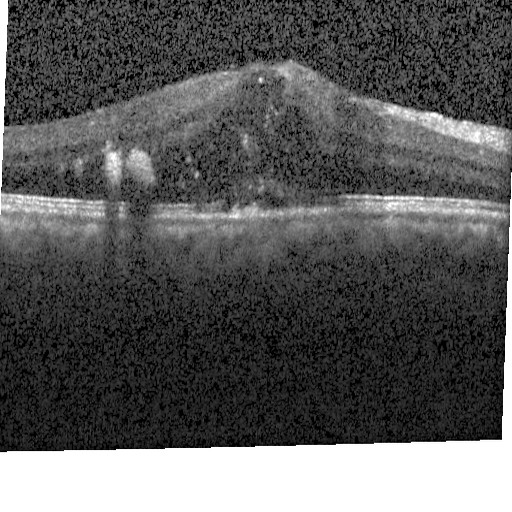
OCT line scan, instrument: Heidelberg Spectralis, spectral-domain OCT — Dx: diabetic macular edema (DME).